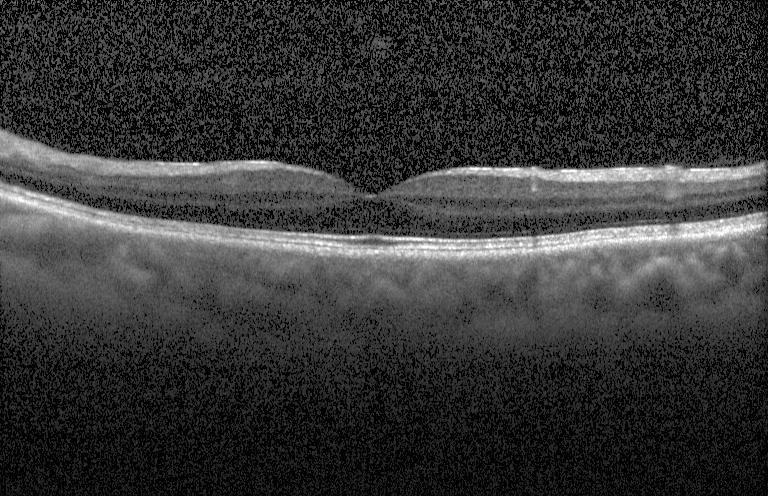
Finding: no evidence of choroidal neovascularization, diabetic macular edema, or drusen.